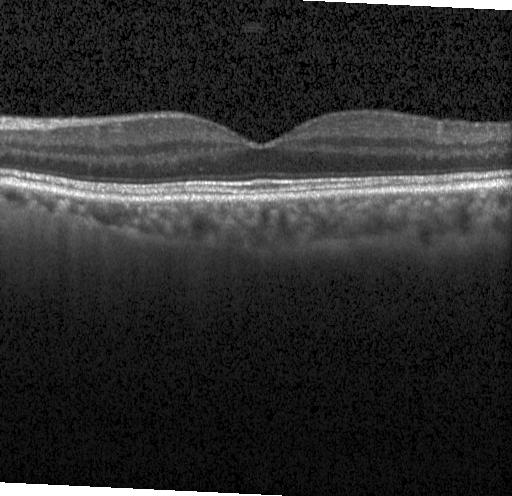 Diagnosis: no choroidal neovascularization, diabetic macular edema, or drusen.